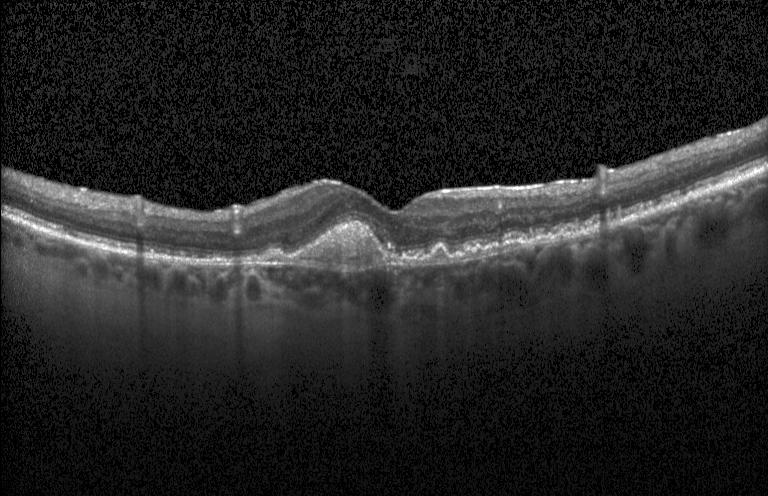
Optical coherence tomography scan. Impression: CNV.